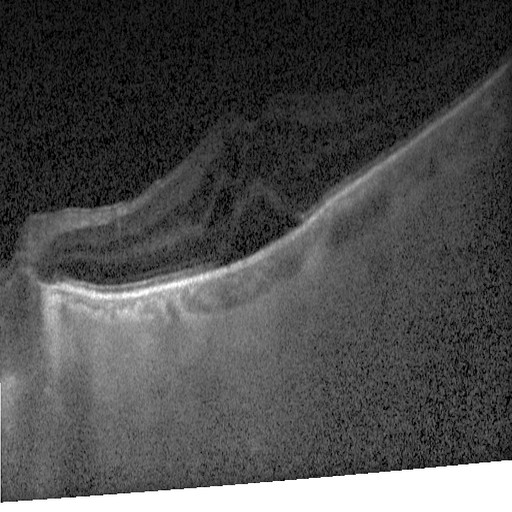 This B-scan demonstrates diabetic macular edema.